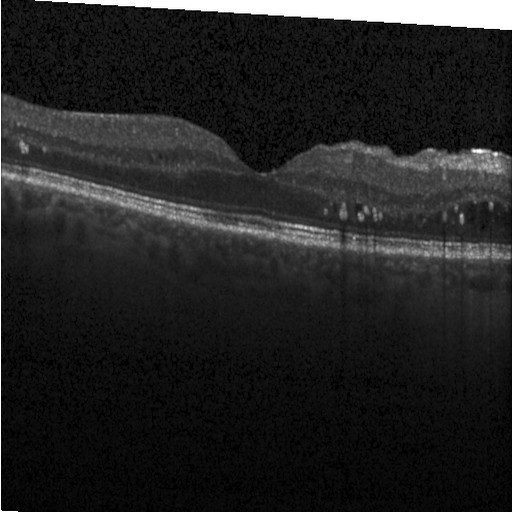
Macular scan · retinal OCT B-scan. Diagnosis: diabetic macular edema.